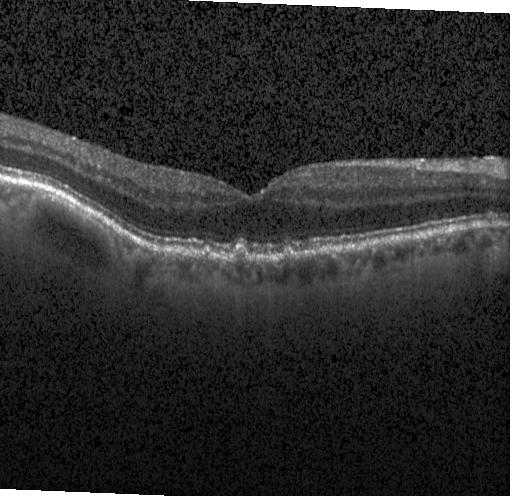

The scan shows drusen.